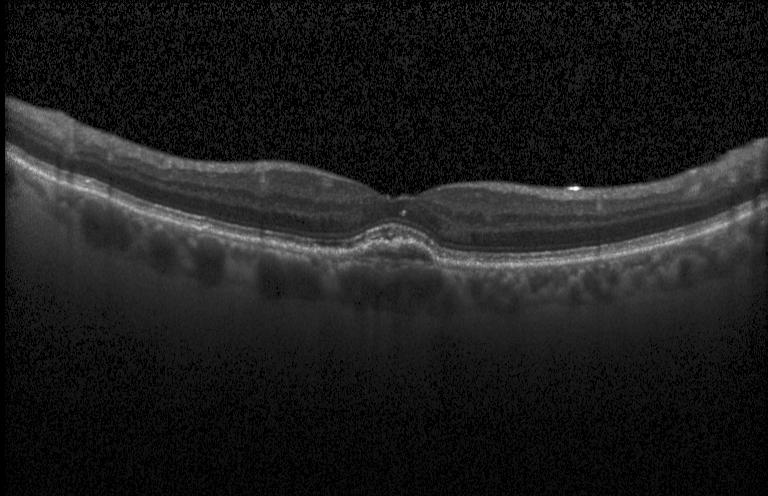
Retinal OCT cross-section · Heidelberg Spectralis
Finding: a choroidal neovascular membrane.